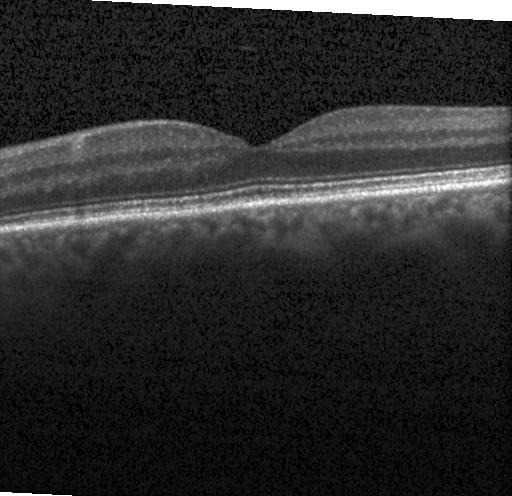

Spectral-domain optical coherence tomography, optical coherence tomography scan
Diagnosis: no choroidal neovascularization, no diabetic macular edema, and no drusen.